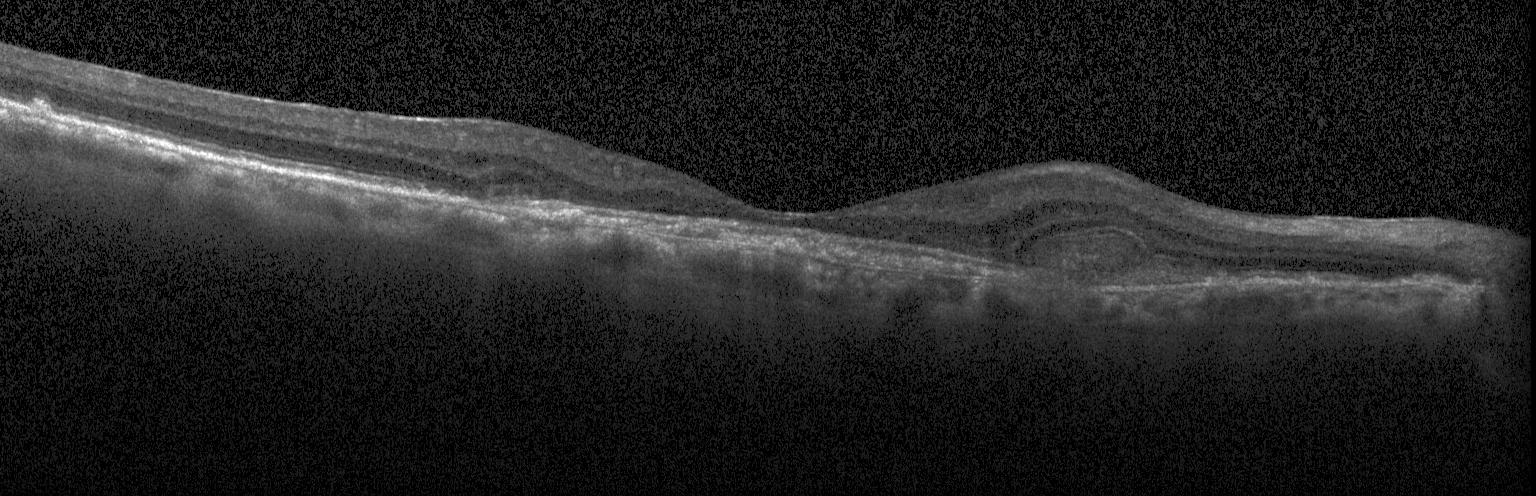
SD-OCT, fovea-centered, Heidelberg Spectralis, retinal OCT cross-section. Finding: choroidal neovascularization (CNV).